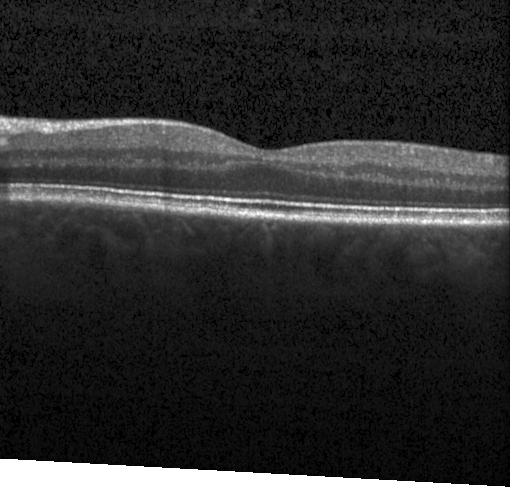 Heidelberg Spectralis; retinal OCT B-scan
Diagnosis: no choroidal neovascularization, diabetic macular edema, or drusen.